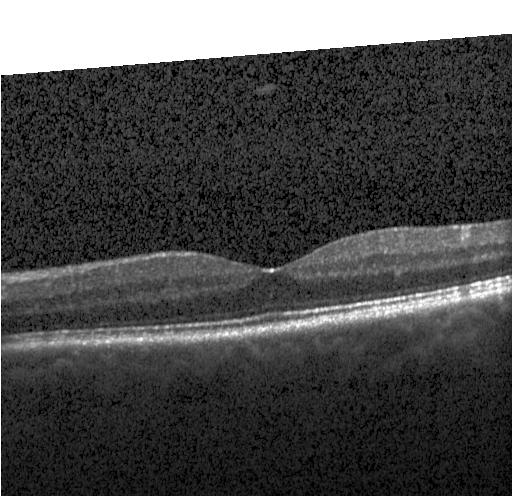

OCT B-scan showing no choroidal neovascularization, no diabetic macular edema, and no drusen.